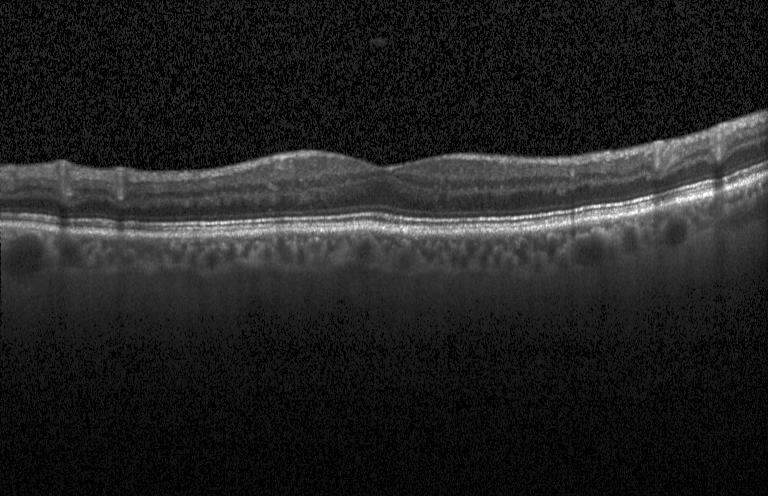

Heidelberg Spectralis OCT system, spectral-domain OCT, retinal OCT cross-section.
Impression: no evidence of CNV, DME, or drusen.